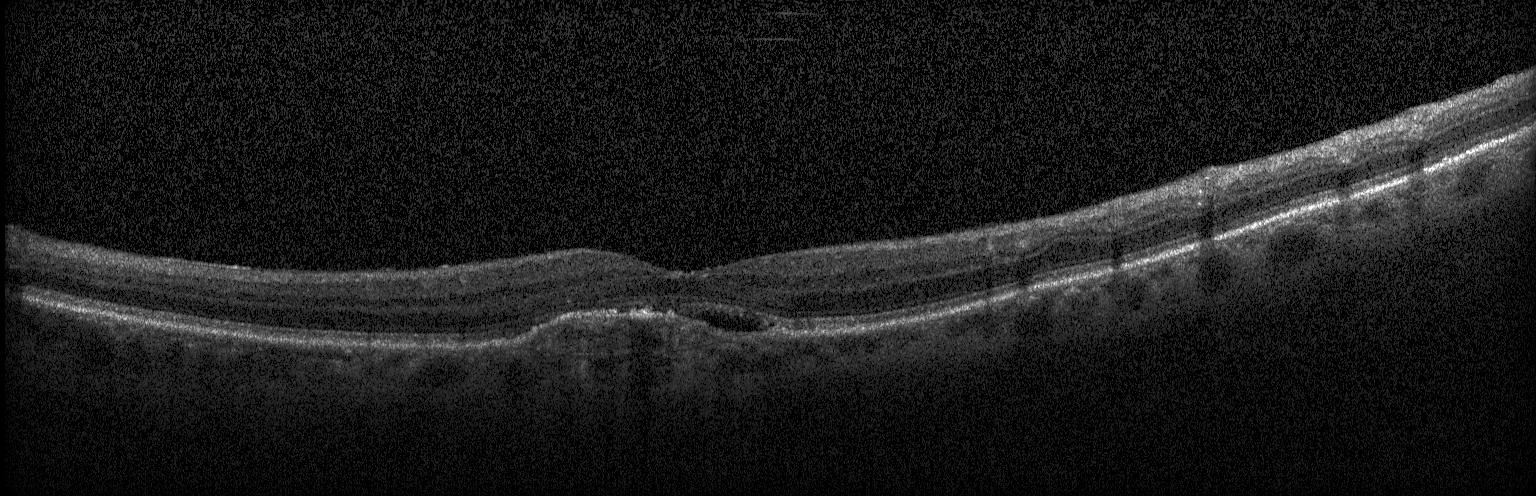 Retinal OCT B-scan. Through the macula. Spectral-domain optical coherence tomography
Diagnosis: choroidal neovascularization.